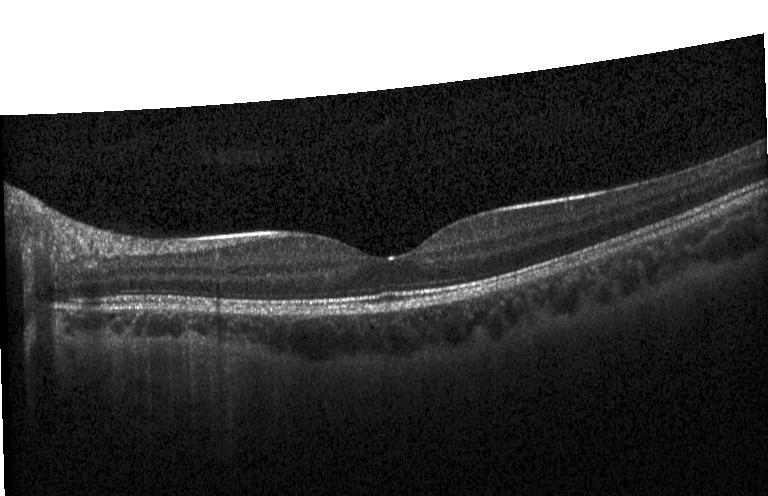 Diagnosis: no evidence of CNV, DME, or drusen.